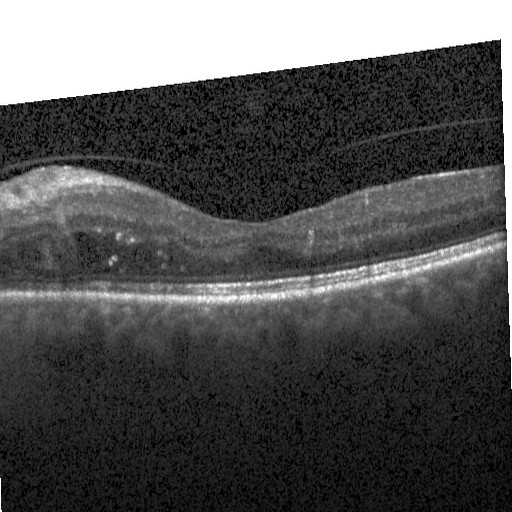

Impression: diabetic macular edema.